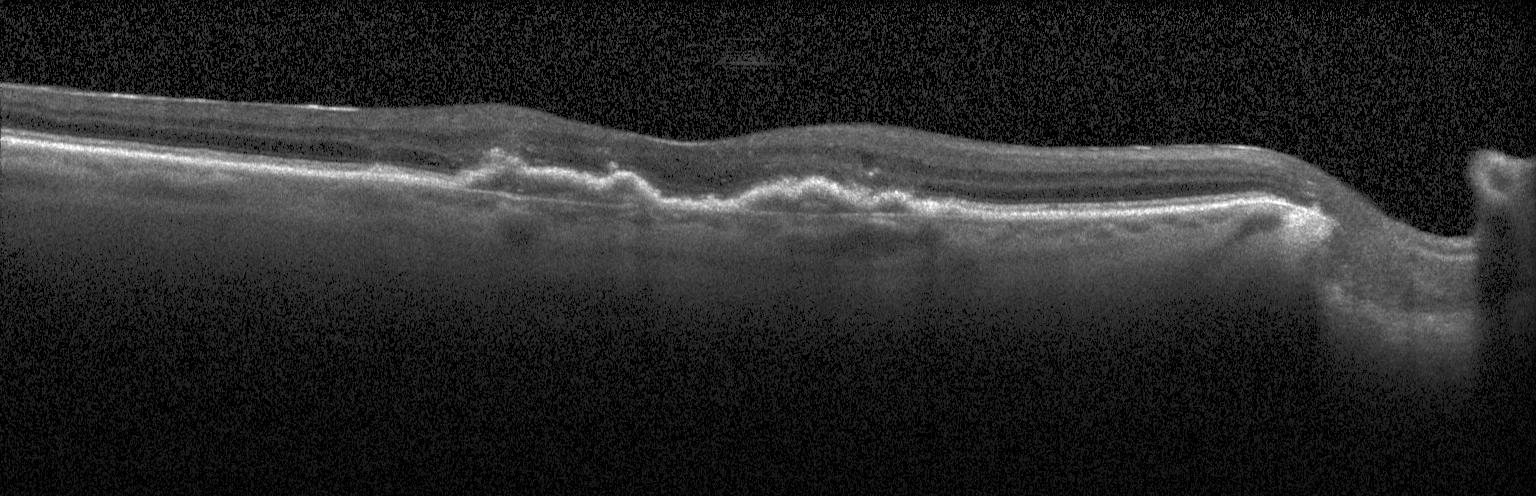

Retinal OCT cross-section showing a choroidal neovascular membrane.